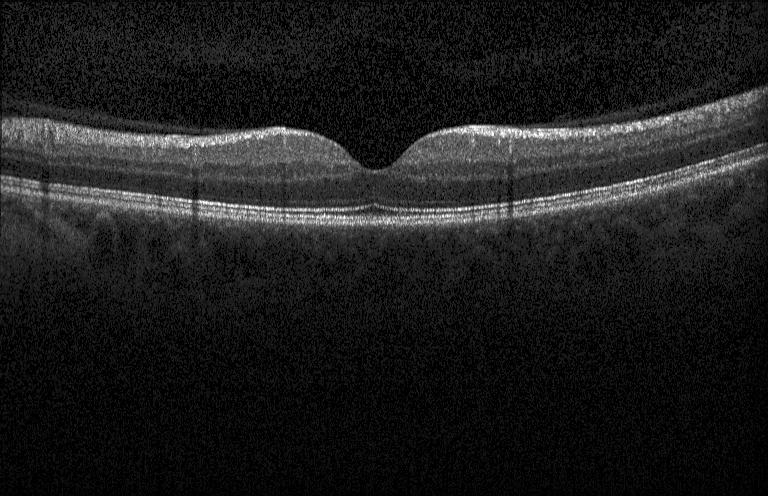 Acquired on a Heidelberg Spectralis · optical coherence tomography B-scan · SD-OCT.
No choroidal neovascularization, no diabetic macular edema, and no drusen.